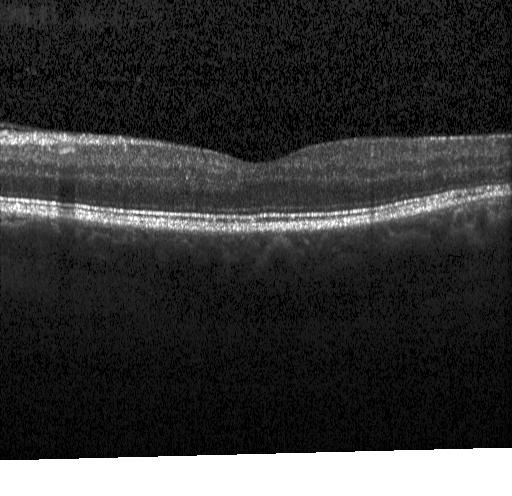
Heidelberg Spectralis. Retinal OCT B-scan
Impression: no choroidal neovascularization, diabetic macular edema, or drusen.